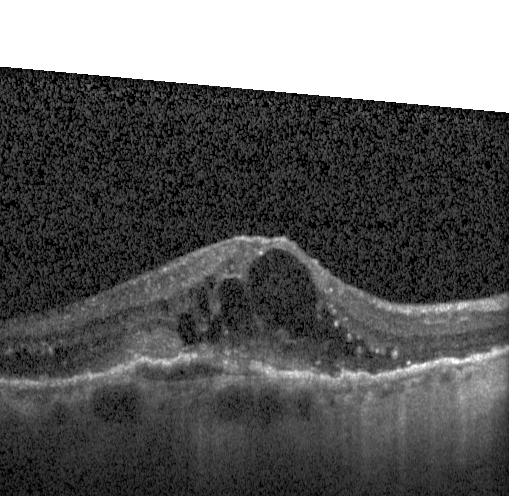 Fovea-centered, optical coherence tomography B-scan, SD-OCT, acquired on a Heidelberg Spectralis
OCT finding: choroidal neovascularization (CNV).